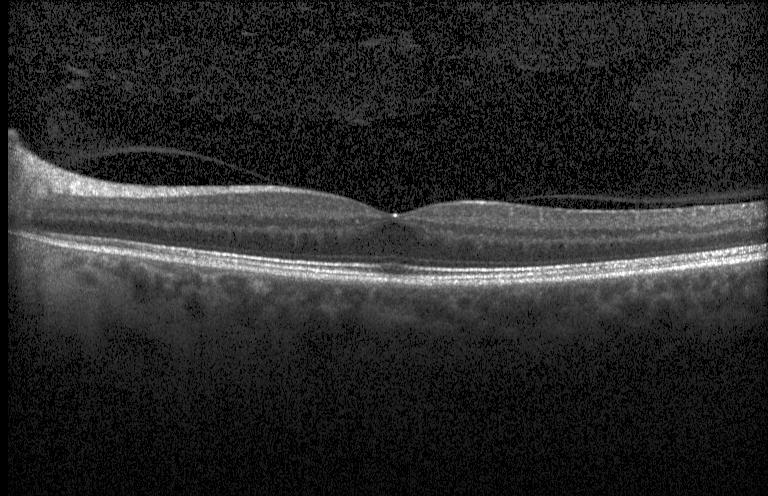

Assessment: no choroidal neovascularization, diabetic macular edema, or drusen.